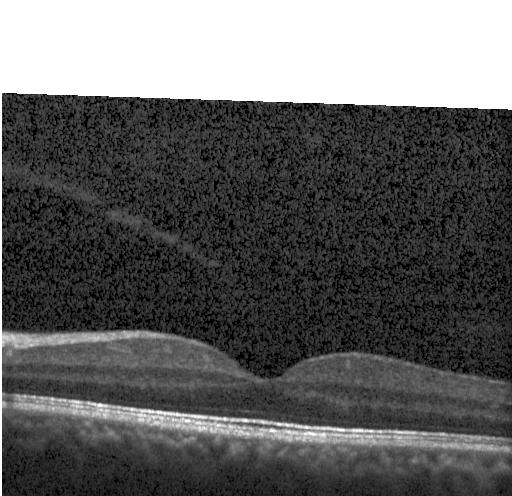

SD-OCT; retinal OCT B-scan. Diagnosis: no choroidal neovascularization, no diabetic macular edema, and no drusen.